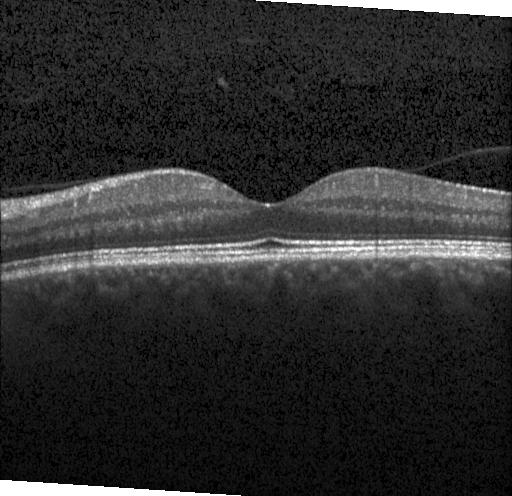 Optical coherence tomography B-scan — Finding: no choroidal neovascularization, diabetic macular edema, or drusen.